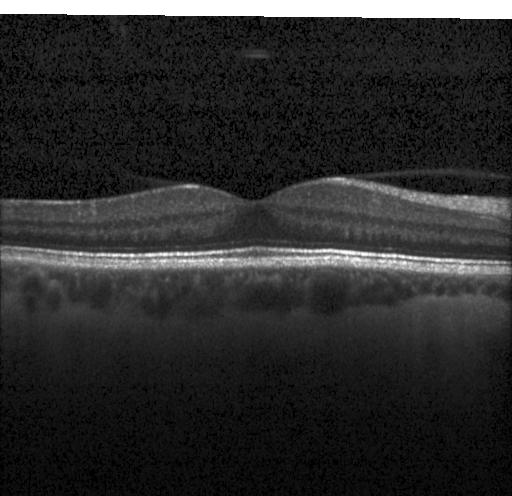

Heidelberg Spectralis OCT system · SD-OCT · macular scan · OCT line scan. Impression: no evidence of choroidal neovascularization, diabetic macular edema, or drusen.